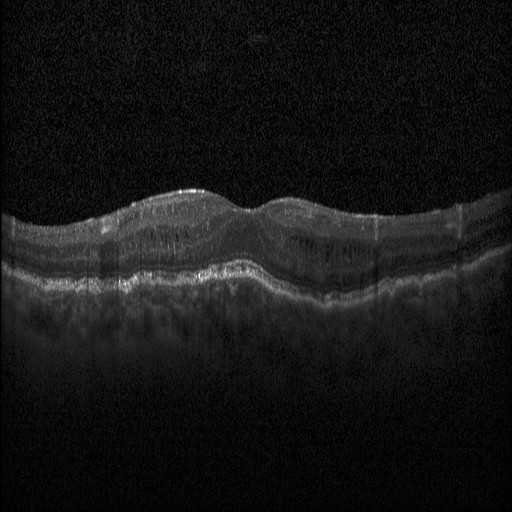

Fovea-centered, retinal OCT B-scan, Heidelberg Spectralis, spectral-domain OCT
Assessment: diabetic macular edema.